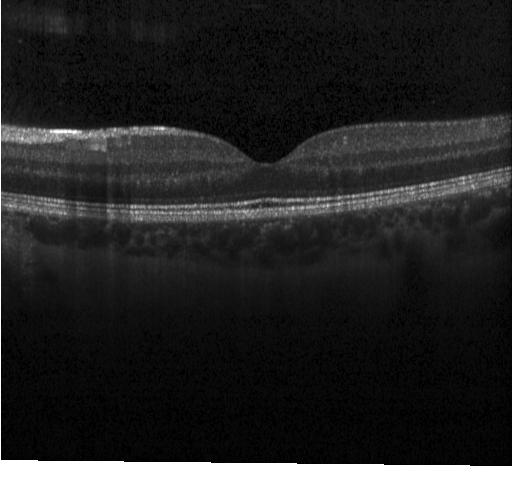
Spectral-domain optical coherence tomography · Heidelberg Spectralis OCT system · retinal OCT cross-section · centered on the fovea.
Impression: no CNV, no DME, and no drusen.